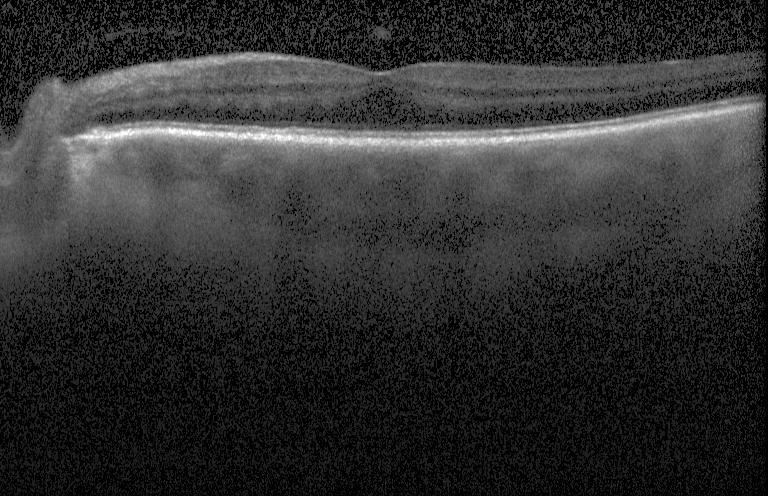
Finding: neither CNV, DME, nor drusen.